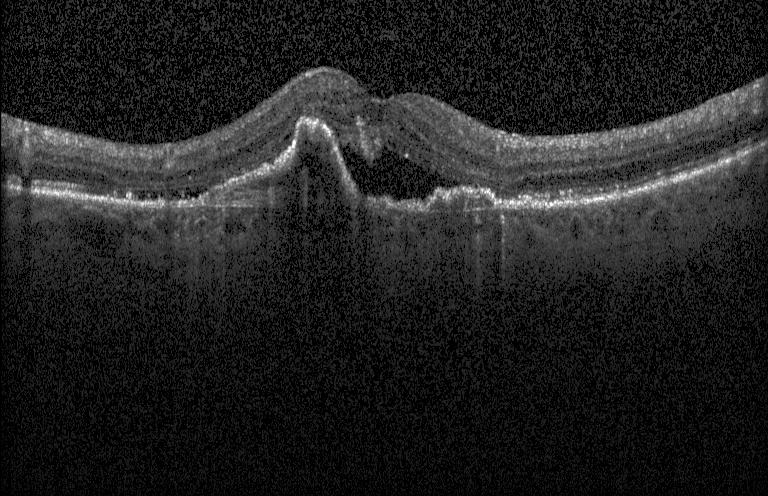

Finding: choroidal neovascularization (CNV).